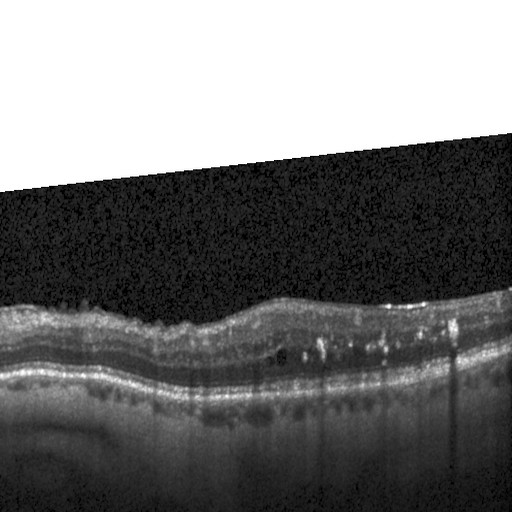
SD-OCT. Retinal OCT cross-section. Assessment: DME.